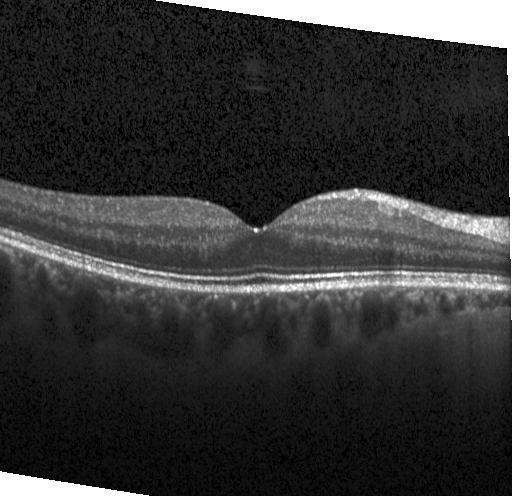
Acquired on a Heidelberg Spectralis, optical coherence tomography B-scan
Impression: no CNV, DME, or drusen.